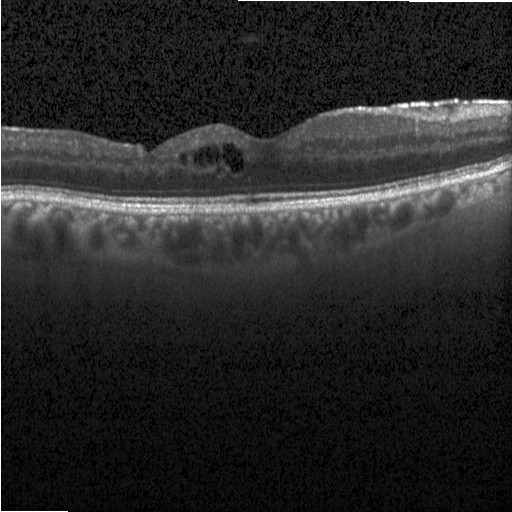 Optical coherence tomography scan · spectral-domain OCT · Heidelberg Spectralis OCT system
The scan shows diabetic macular edema (DME).